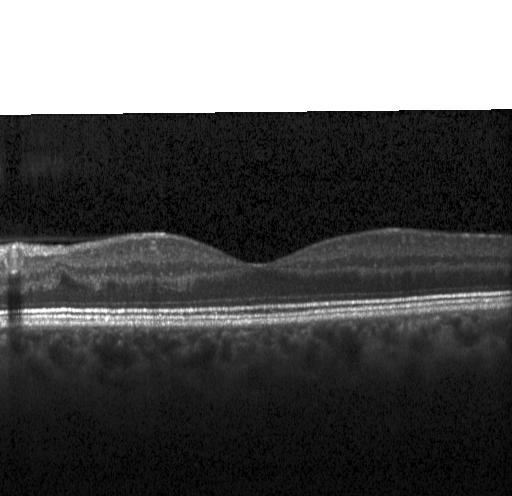

Retinal OCT B-scan — OCT finding: neither choroidal neovascularization, diabetic macular edema, nor drusen.